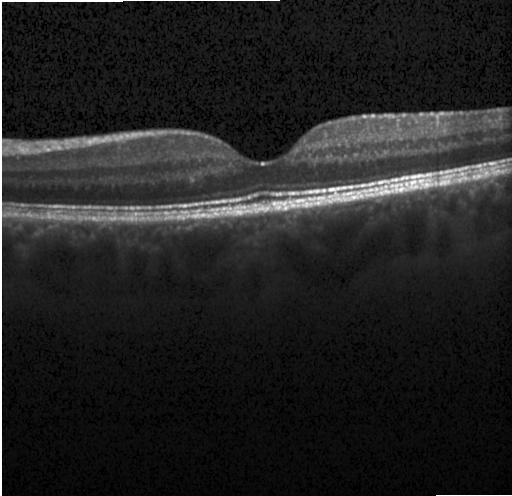
OCT finding: no evidence of choroidal neovascularization, diabetic macular edema, or drusen.